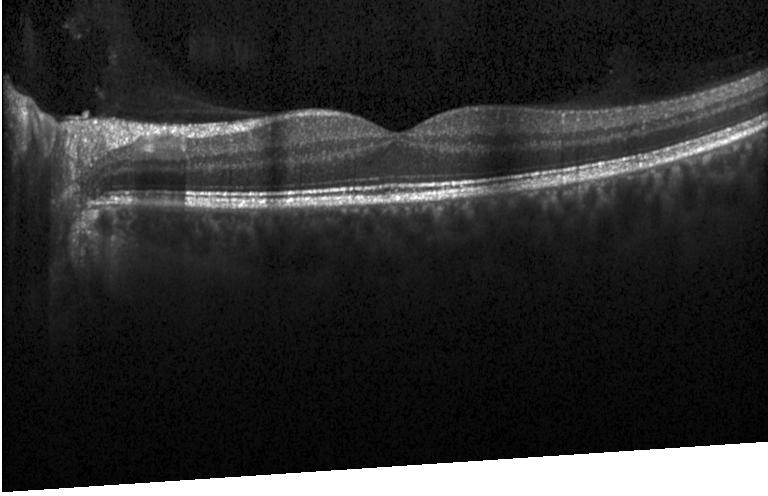 Optical coherence tomography scan. Dx: neither CNV, DME, nor drusen.